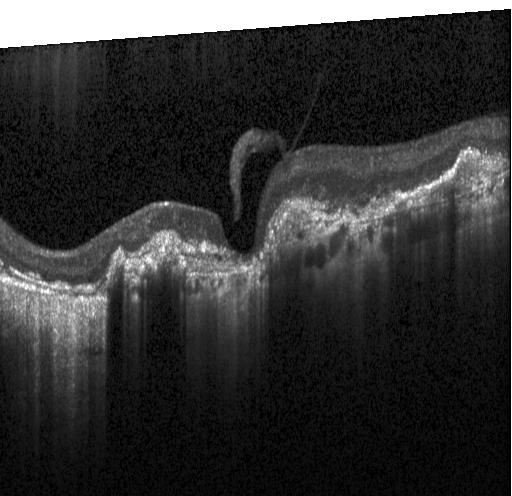
Optical coherence tomography B-scan; SD-OCT.
Dx: CNV.